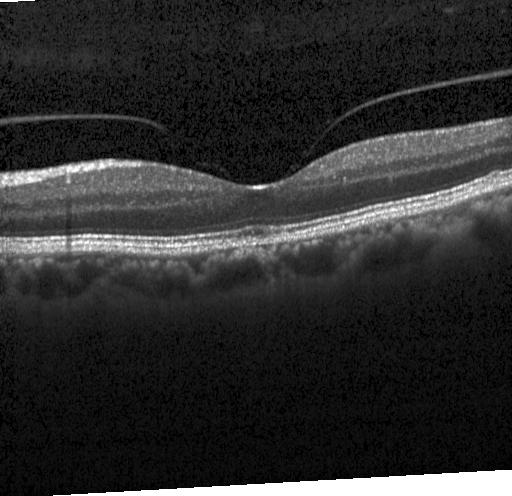
OCT line scan, macular scan, spectral-domain OCT. Dx: no evidence of choroidal neovascularization, diabetic macular edema, or drusen.